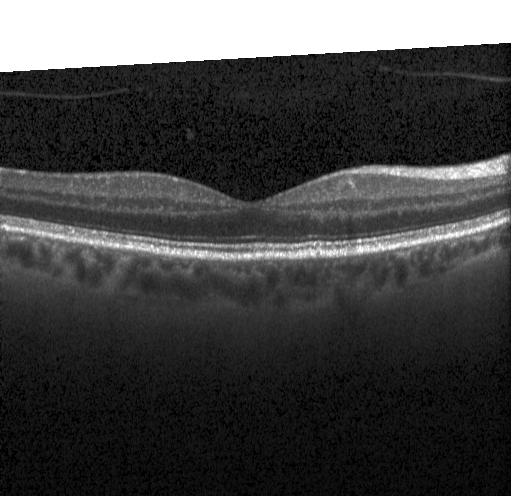

Acquired on a Heidelberg Spectralis · horizontal scan through the fovea · SD-OCT · OCT B-scan. Dx: no choroidal neovascularization, diabetic macular edema, or drusen.